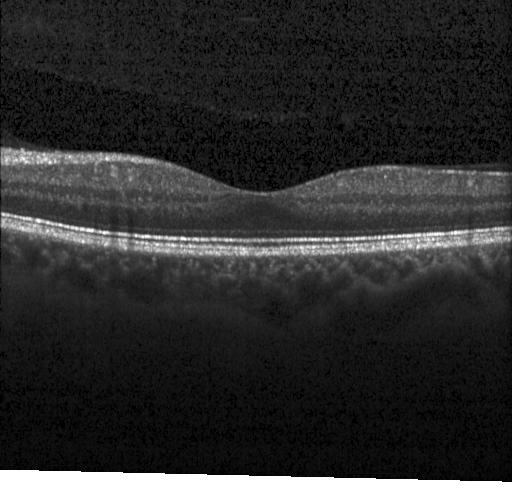
The scan shows no evidence of choroidal neovascularization, diabetic macular edema, or drusen.